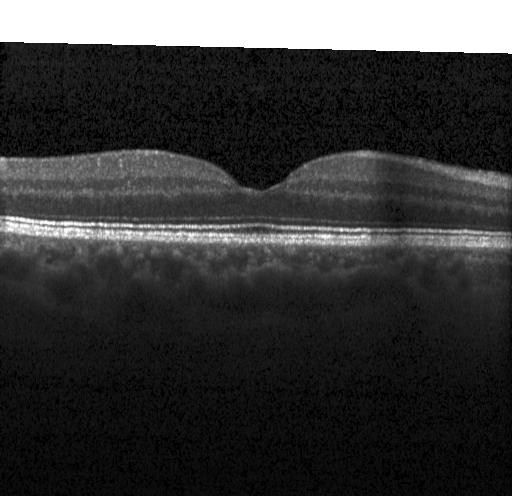
Retinal OCT cross-section — Dx: no choroidal neovascularization, diabetic macular edema, or drusen.